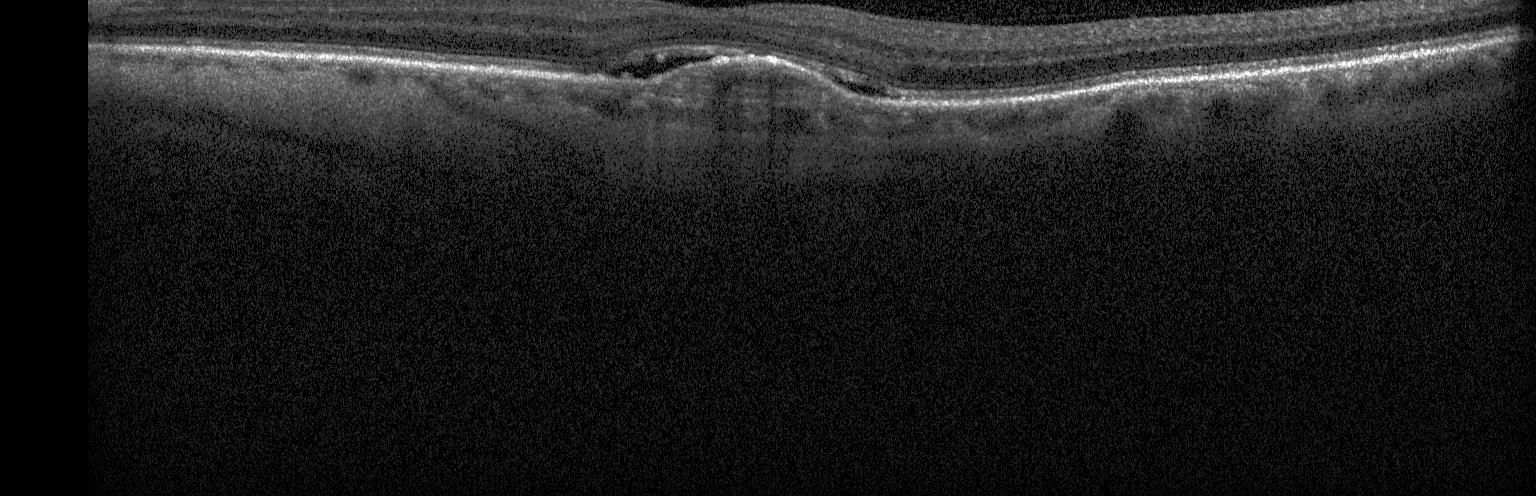
SD-OCT · retinal OCT B-scan — This B-scan demonstrates choroidal neovascularization.